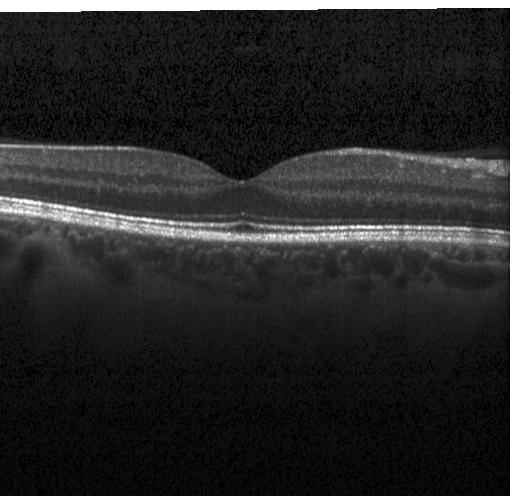

OCT scan showing no evidence of choroidal neovascularization, diabetic macular edema, or drusen.